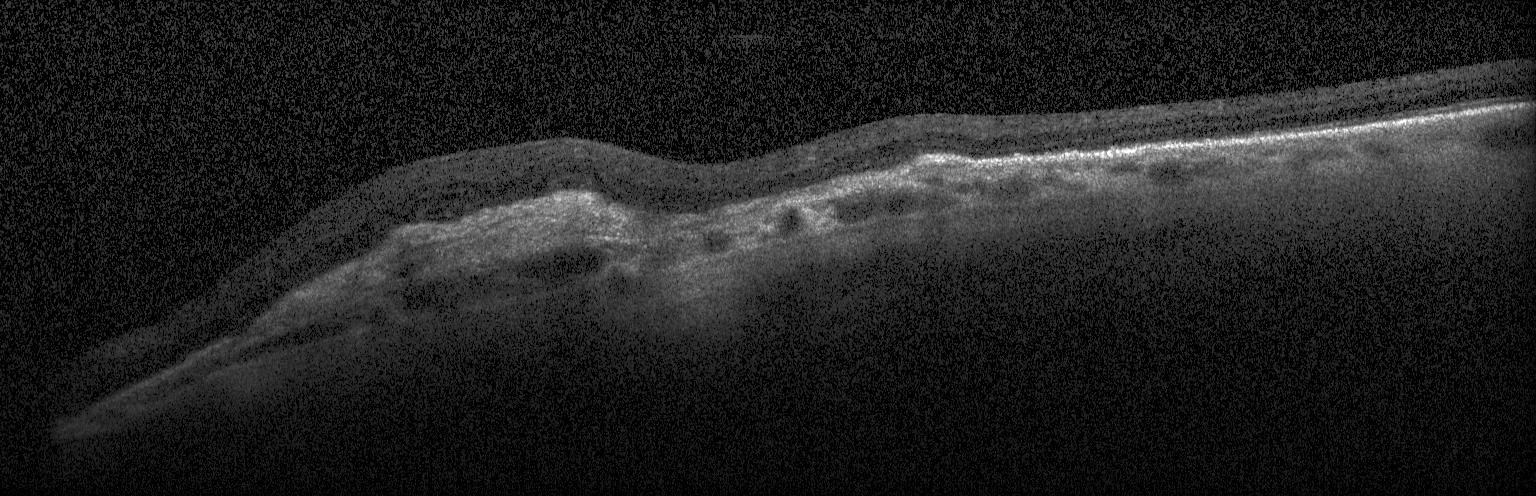

Heidelberg Spectralis; OCT line scan; horizontal scan through the fovea.
This B-scan demonstrates CNV.